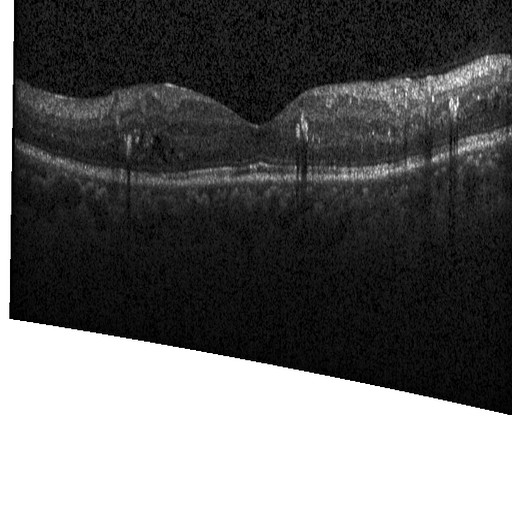

Heidelberg Spectralis; horizontal scan through the fovea; optical coherence tomography scan; SD-OCT.
Impression: diabetic macular edema.